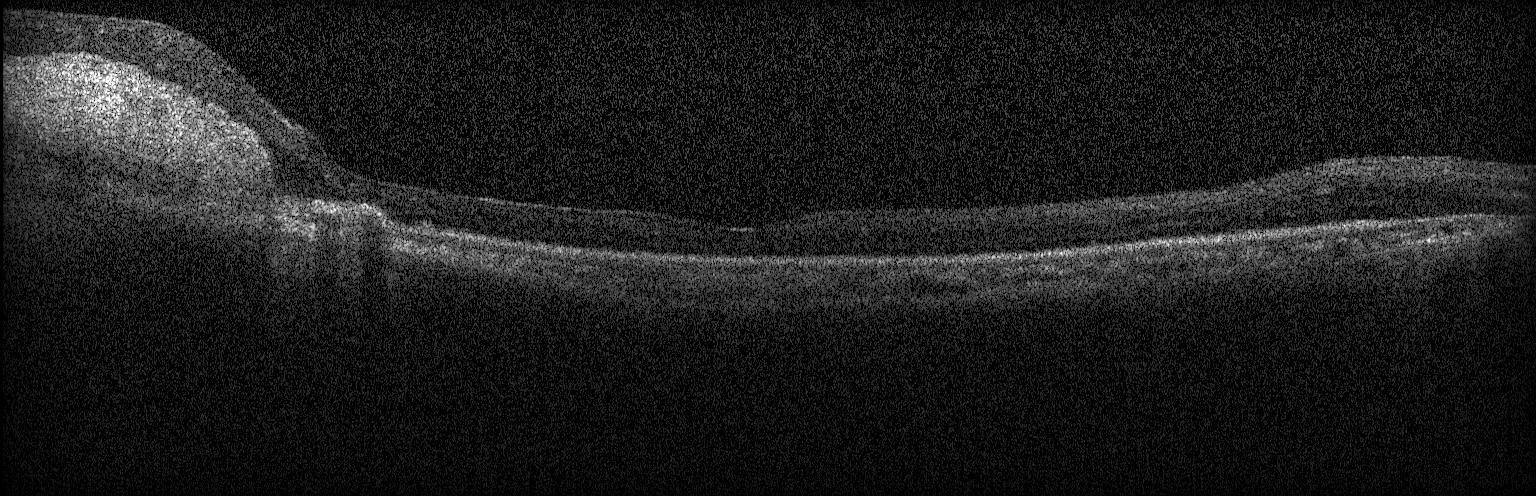 Dx: choroidal neovascularization.